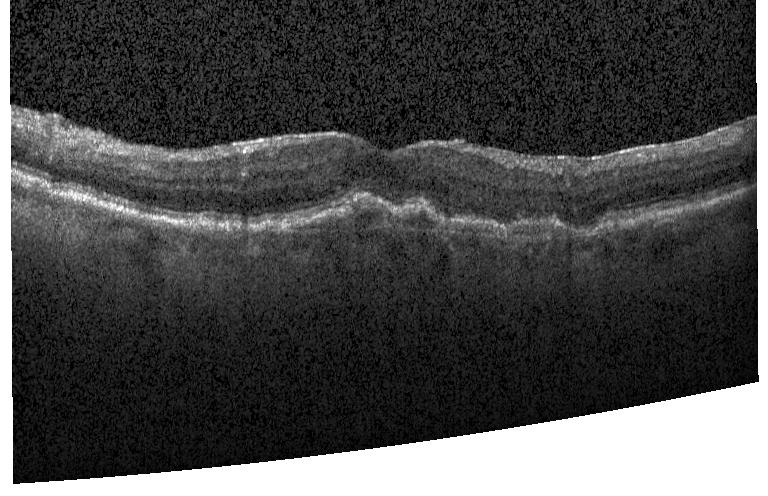 Optical coherence tomography B-scan
Diagnosis: CNV.